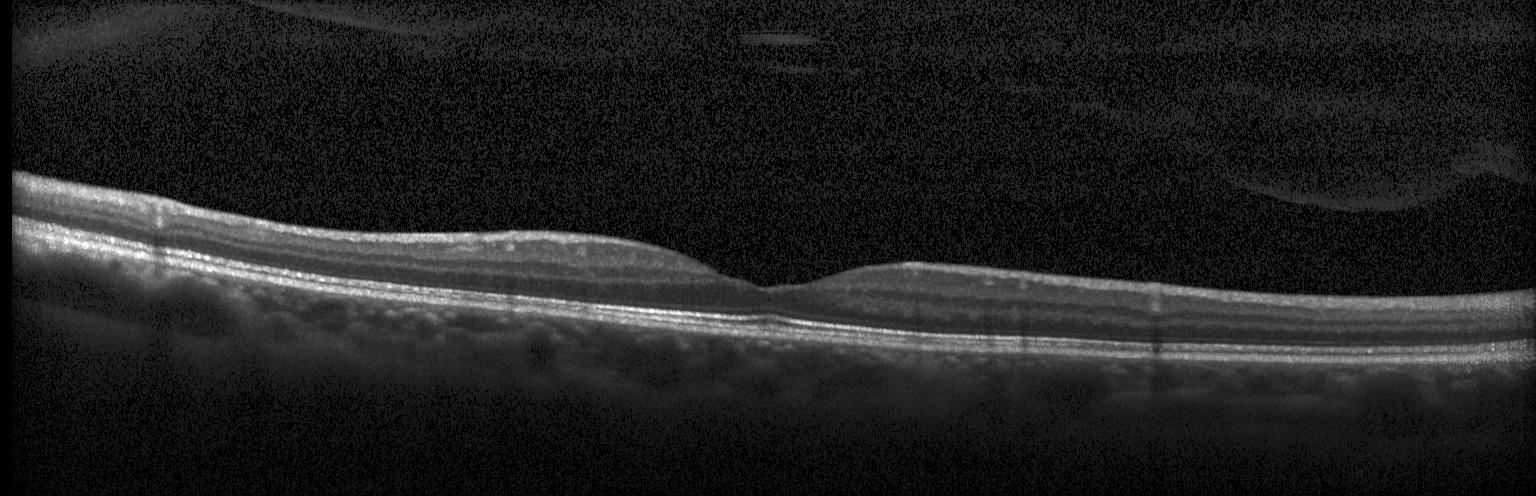

Optical coherence tomography B-scan. Acquired on a Heidelberg Spectralis. No evidence of choroidal neovascularization, diabetic macular edema, or drusen.